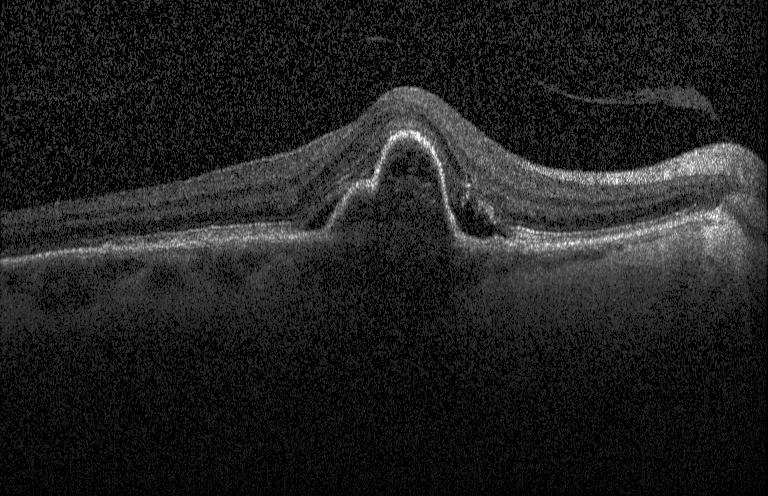 OCT B-scan. Macular scan. Heidelberg Spectralis. Spectral-domain optical coherence tomography
Diagnosis: CNV.